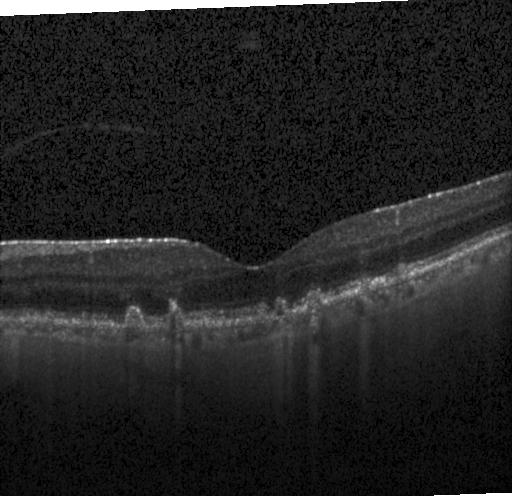 Spectral-domain OCT B-scan: sub-RPE drusenoid deposits.